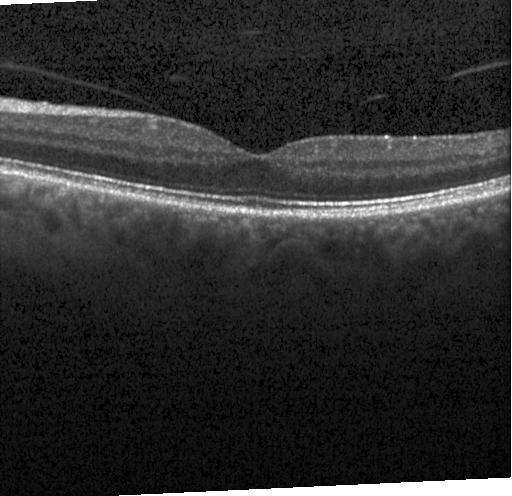

Optical coherence tomography B-scan — No CNV, DME, or drusen.